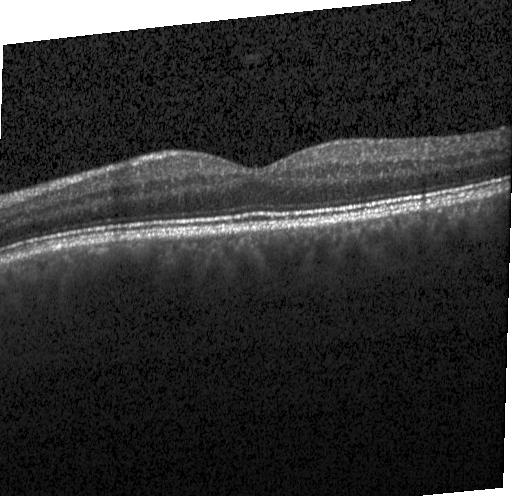

OCT line scan. Spectral-domain OCT — Assessment: no CNV, DME, or drusen.